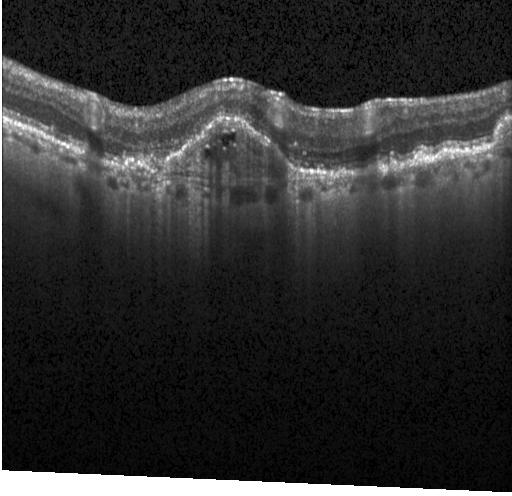
Acquired on a Heidelberg Spectralis, spectral-domain optical coherence tomography, optical coherence tomography B-scan — Assessment: choroidal neovascularization (CNV).